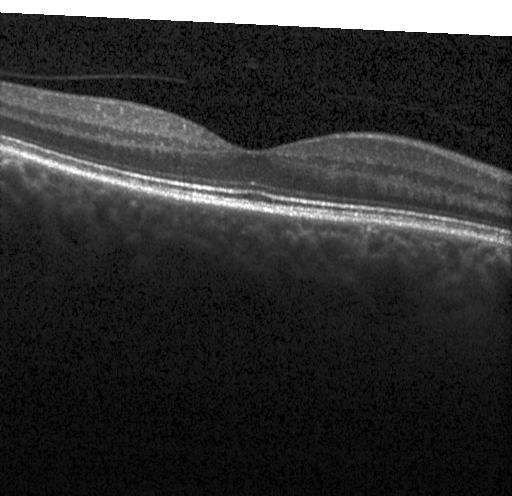

Retinal OCT cross-section
Dx: no evidence of choroidal neovascularization, diabetic macular edema, or drusen.